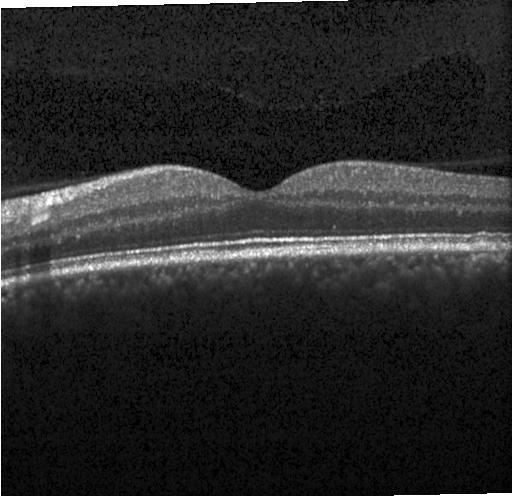

Diagnosis: no evidence of CNV, DME, or drusen.